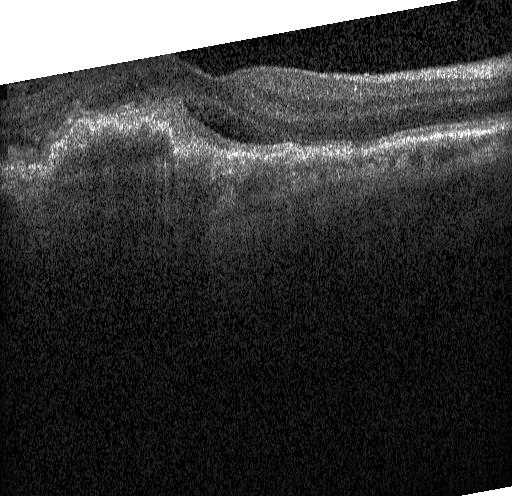 Optical coherence tomography B-scan · spectral-domain optical coherence tomography. Impression: CNV.